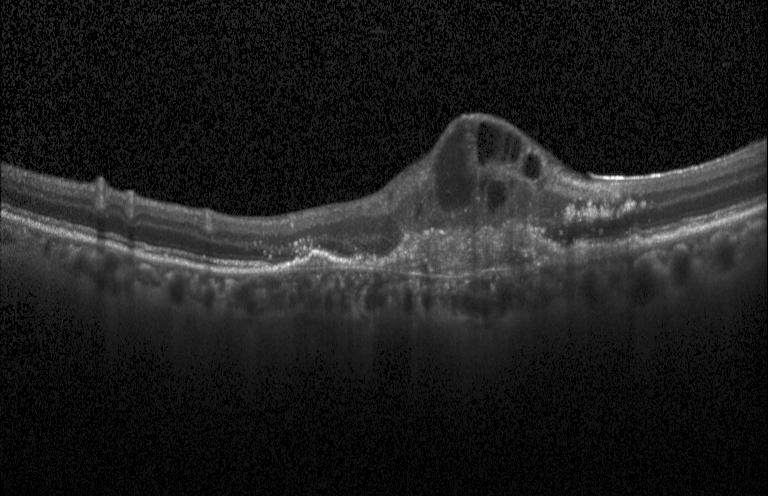
Heidelberg Spectralis OCT system; SD-OCT; fovea-centered; retinal OCT B-scan — Finding: choroidal neovascularization (CNV).